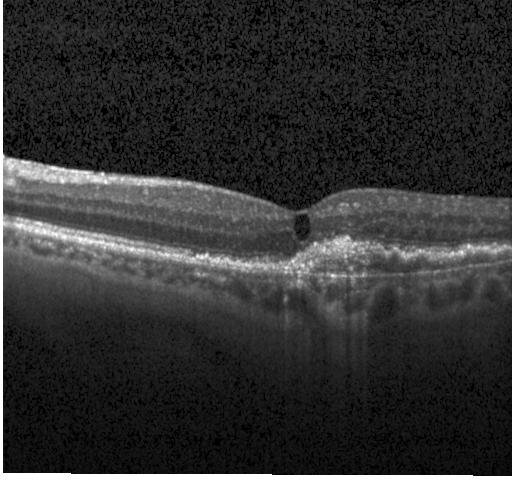
Dx: a choroidal neovascular membrane.